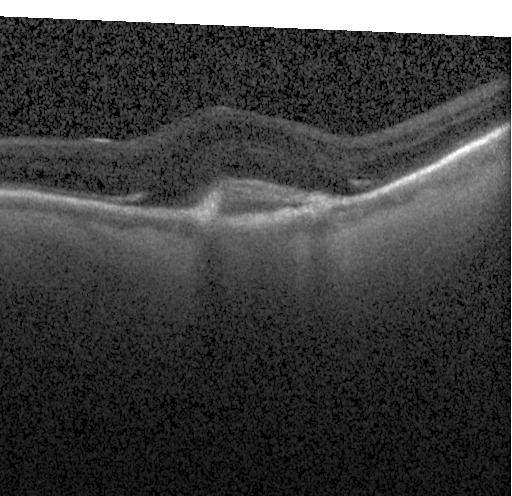
OCT line scan, horizontal scan through the fovea, Heidelberg Spectralis
Finding: choroidal neovascularization (CNV).